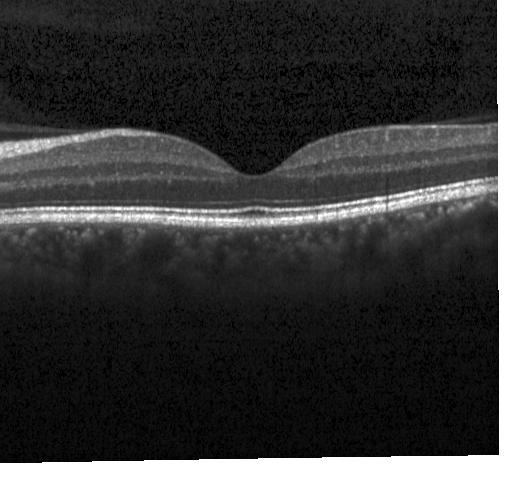
OCT B-scan, centered on the fovea, SD-OCT, acquired on a Heidelberg Spectralis.
Impression: no choroidal neovascularization, no diabetic macular edema, and no drusen.